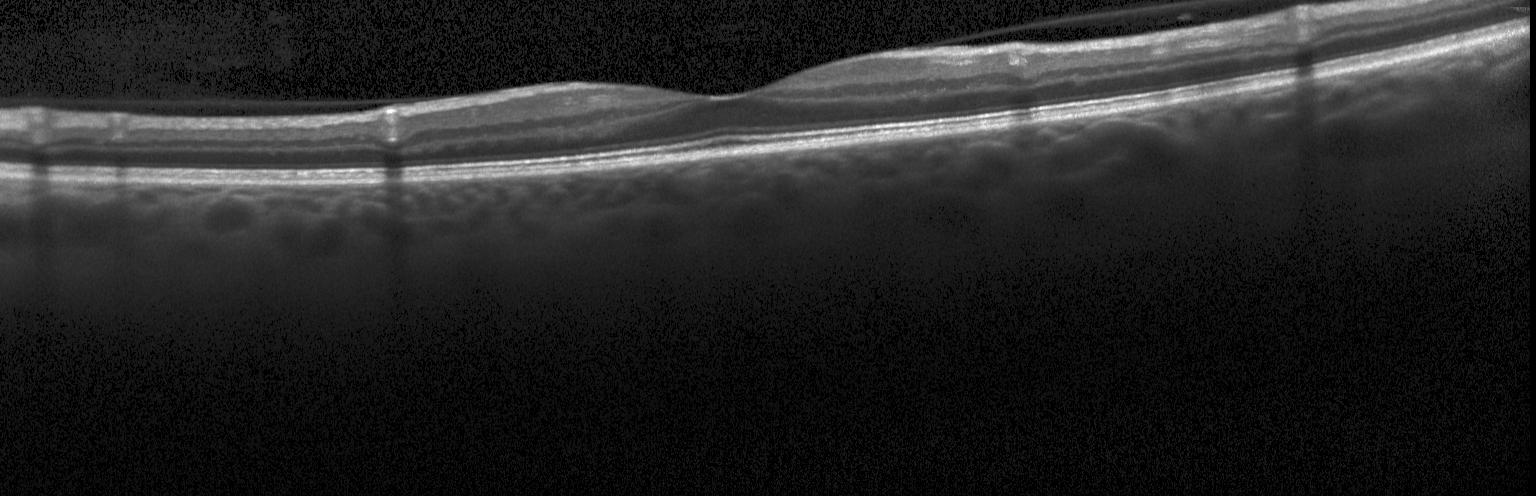
Optical coherence tomography scan
Macular OCT: no evidence of choroidal neovascularization, diabetic macular edema, or drusen.